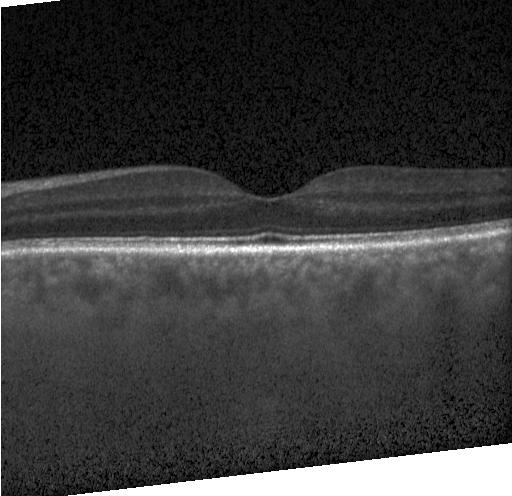

Retinal OCT cross-section; SD-OCT; through the macula — The scan shows no CNV, DME, or drusen.